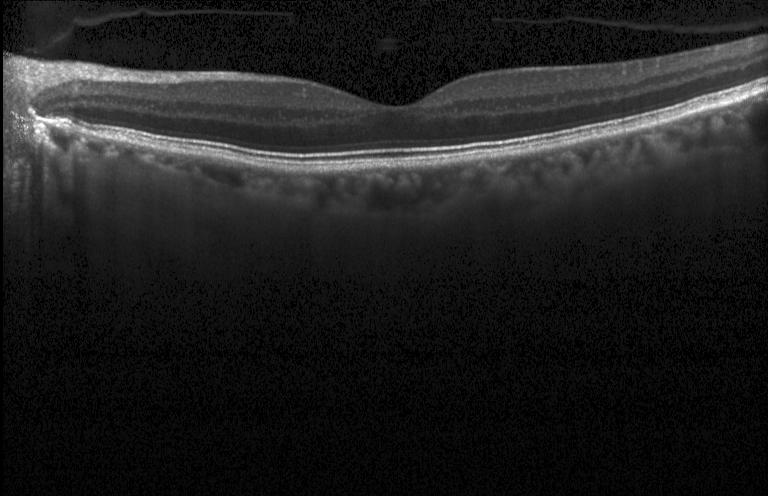
Horizontal scan through the fovea. Retinal OCT cross-section. Spectral-domain OCT. Instrument: Heidelberg Spectralis.
Diagnosis: no choroidal neovascularization, no diabetic macular edema, and no drusen.